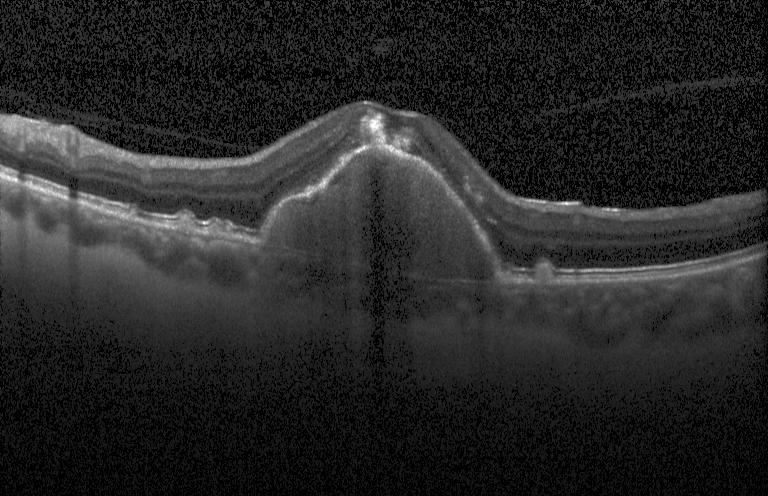 Diagnosis: a choroidal neovascular membrane.